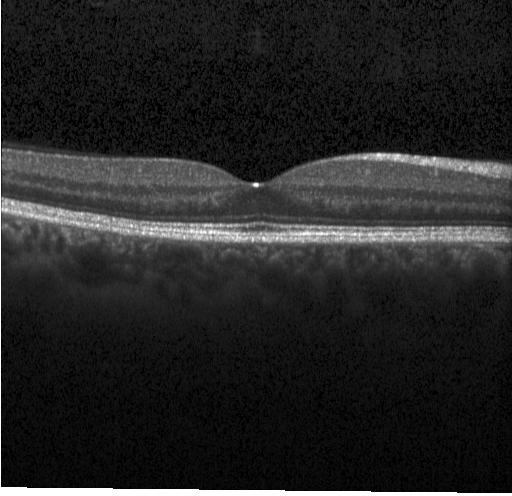 Fovea-centered. Optical coherence tomography B-scan. Heidelberg Spectralis OCT system. Spectral-domain OCT — Assessment: neither CNV, DME, nor drusen.